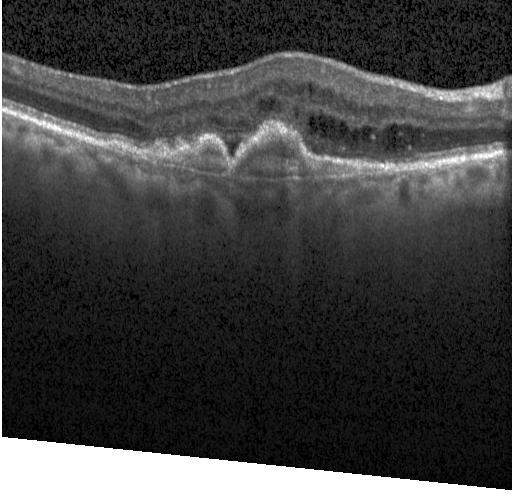

OCT B-scan showing a choroidal neovascular membrane.